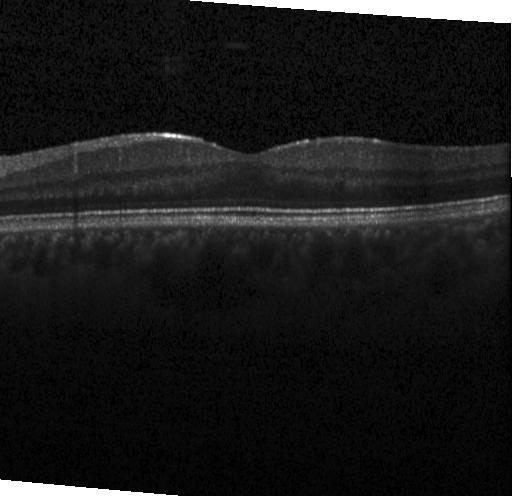 Finding: no CNV, DME, or drusen.